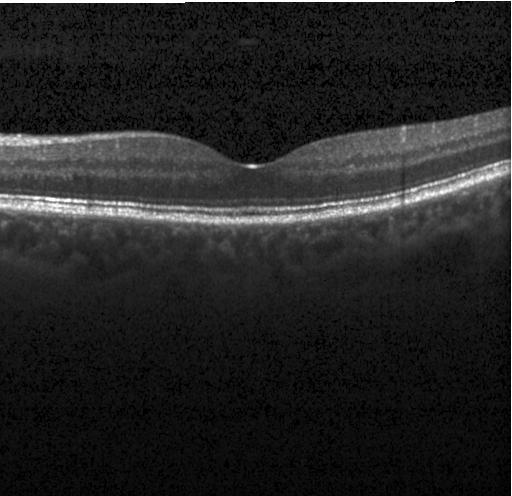

Retinal OCT B-scan
Impression: no choroidal neovascularization, no diabetic macular edema, and no drusen.